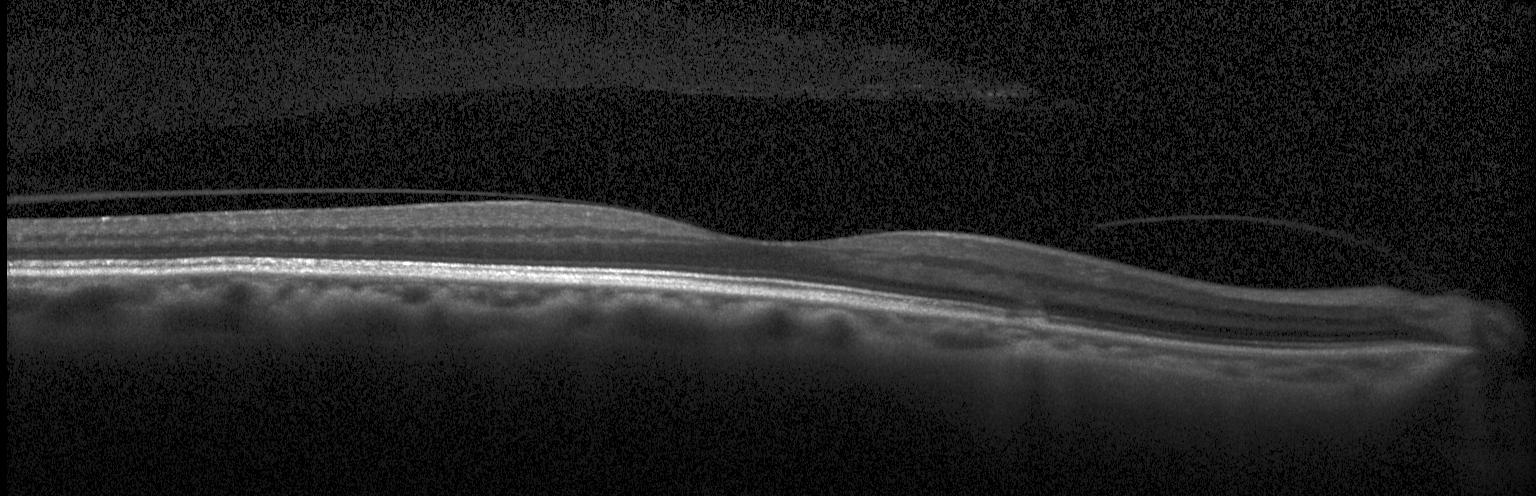 Impression: neither choroidal neovascularization, diabetic macular edema, nor drusen.